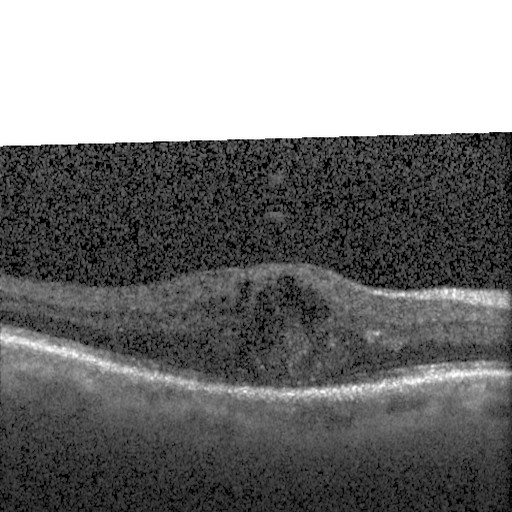

Macular OCT: diabetic macular edema (DME).